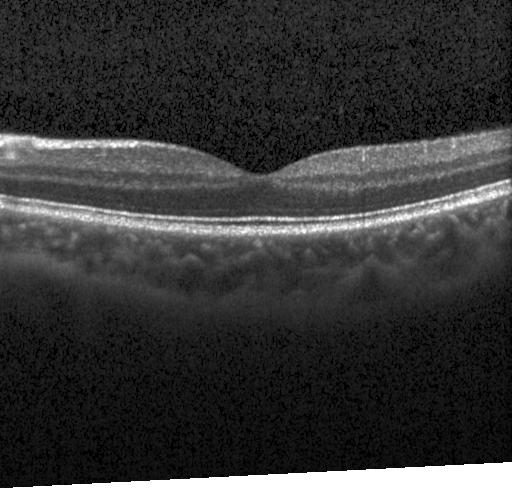
OCT B-scan. Fovea-centered. Acquired on a Heidelberg Spectralis. Spectral-domain OCT — Diagnosis: no evidence of choroidal neovascularization, diabetic macular edema, or drusen.